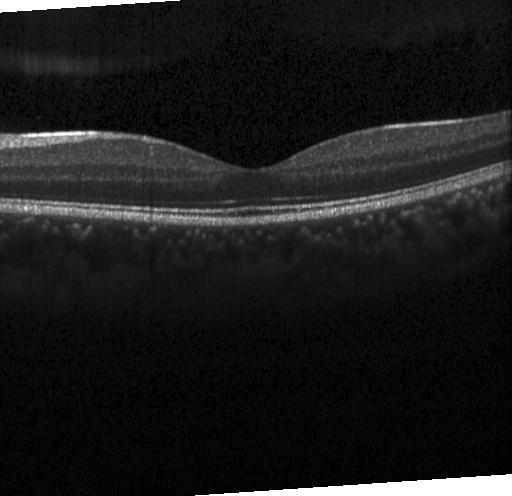

Optical coherence tomography B-scan; fovea-centered; spectral-domain OCT; instrument: Heidelberg Spectralis — This B-scan demonstrates neither CNV, DME, nor drusen.